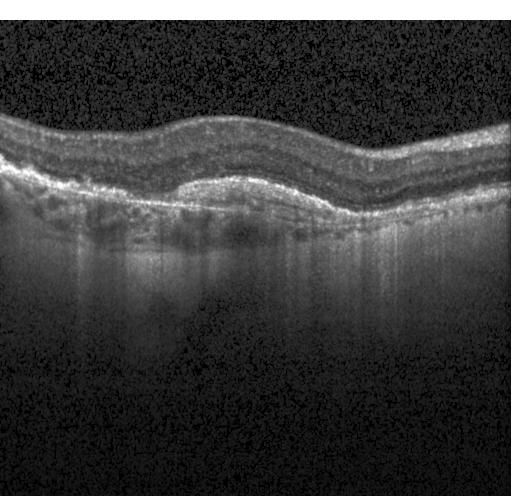 Heidelberg Spectralis, fovea-centered, optical coherence tomography scan. A choroidal neovascular membrane.